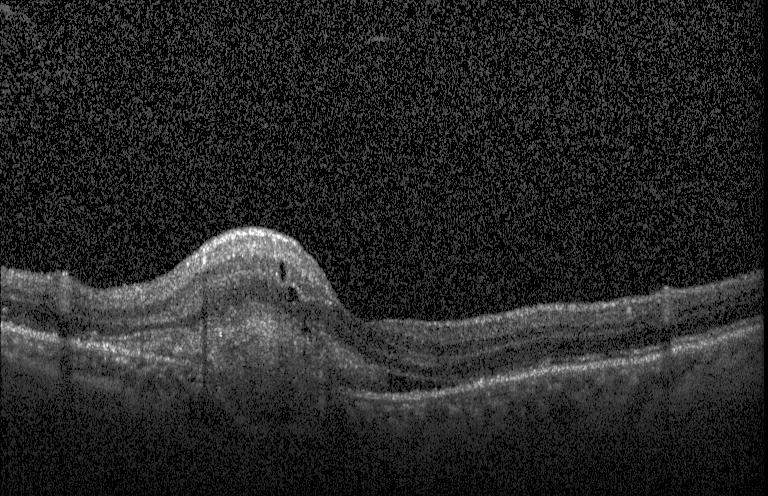

OCT scan showing choroidal neovascularization.